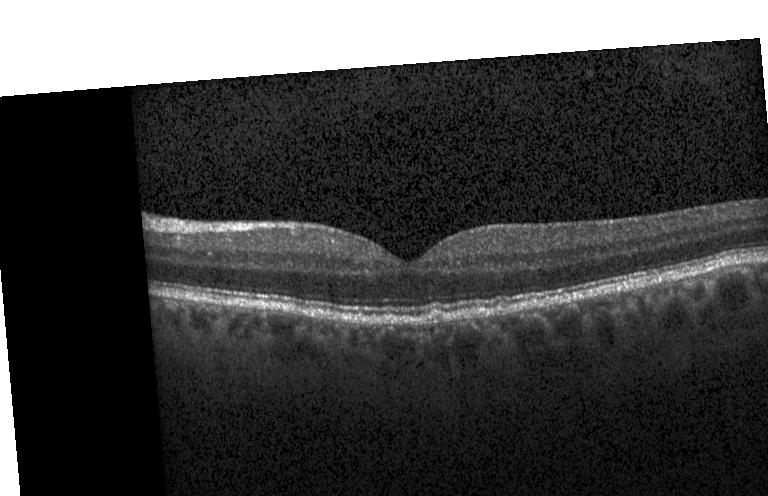 Centered on the fovea. Heidelberg Spectralis. Retinal OCT B-scan — This B-scan demonstrates multiple drusen.